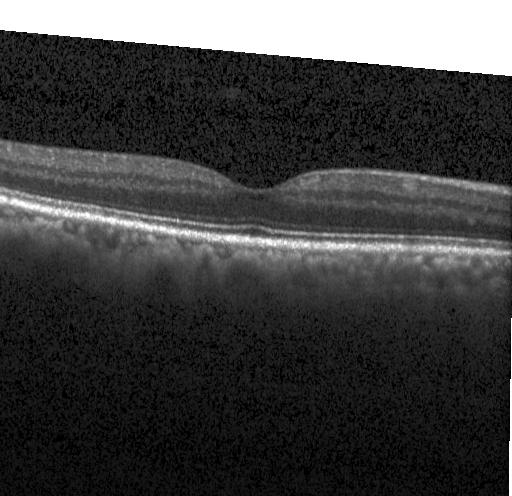 Heidelberg Spectralis OCT system · OCT line scan · spectral-domain OCT
Finding: no choroidal neovascularization, diabetic macular edema, or drusen.